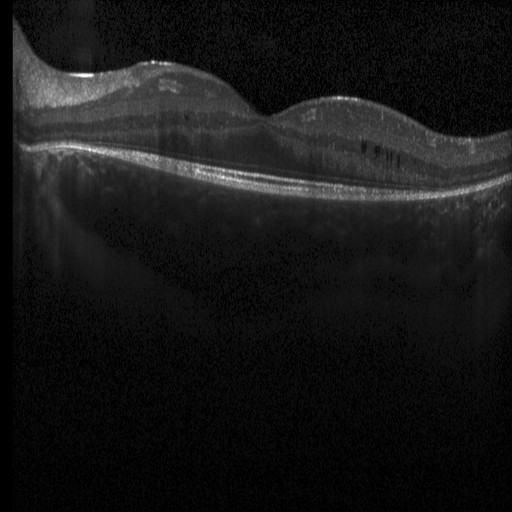

Horizontal scan through the fovea. OCT B-scan.
Macular OCT: DME.